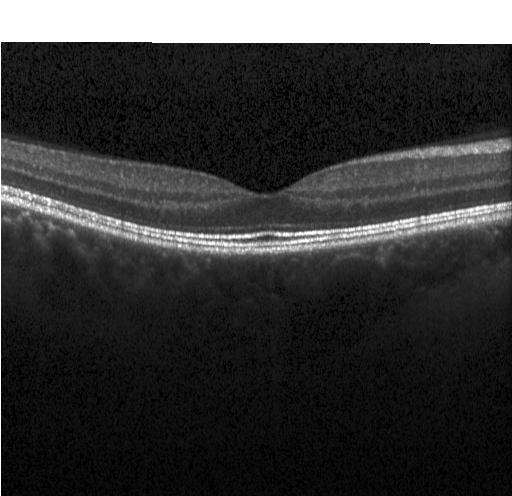 Heidelberg Spectralis OCT system. OCT line scan. Centered on the fovea
Impression: no choroidal neovascularization, diabetic macular edema, or drusen.